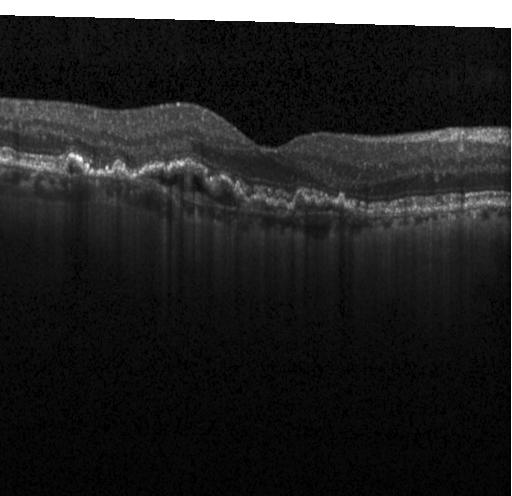

Diagnosis: a choroidal neovascular membrane.